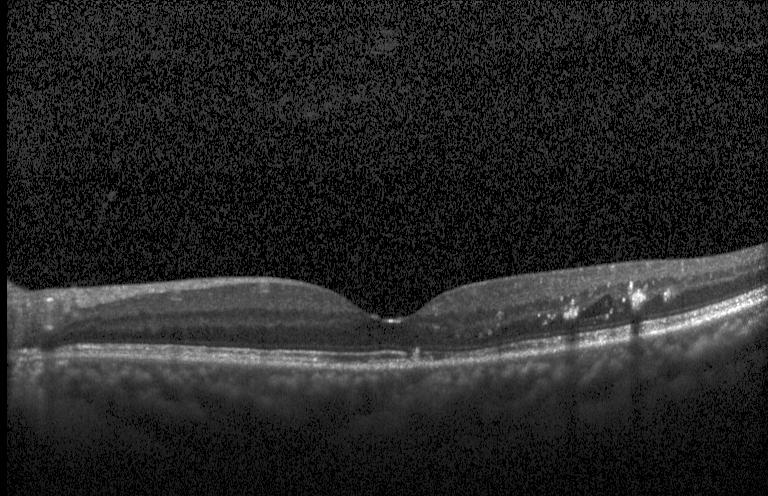 Through the macula; spectral-domain OCT; Heidelberg Spectralis; retinal OCT B-scan — Diagnosis: DME.